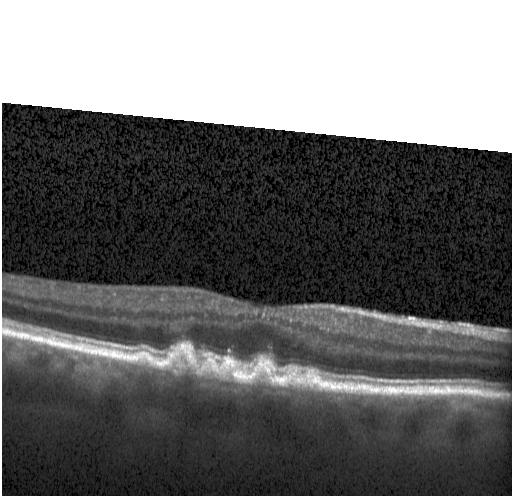
Spectral-domain optical coherence tomography. Optical coherence tomography scan.
The scan shows multiple drusen.